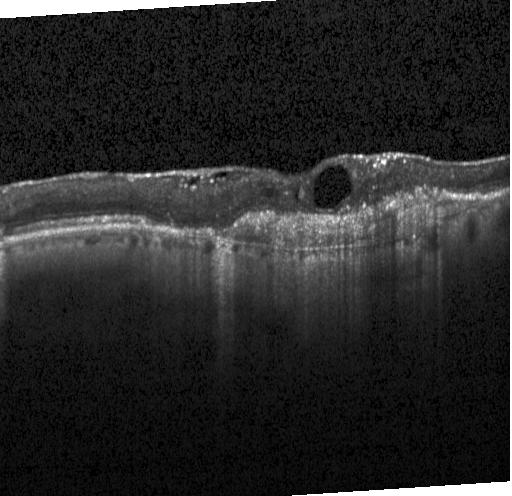
Macular scan · Heidelberg Spectralis · optical coherence tomography scan
Finding: CNV.